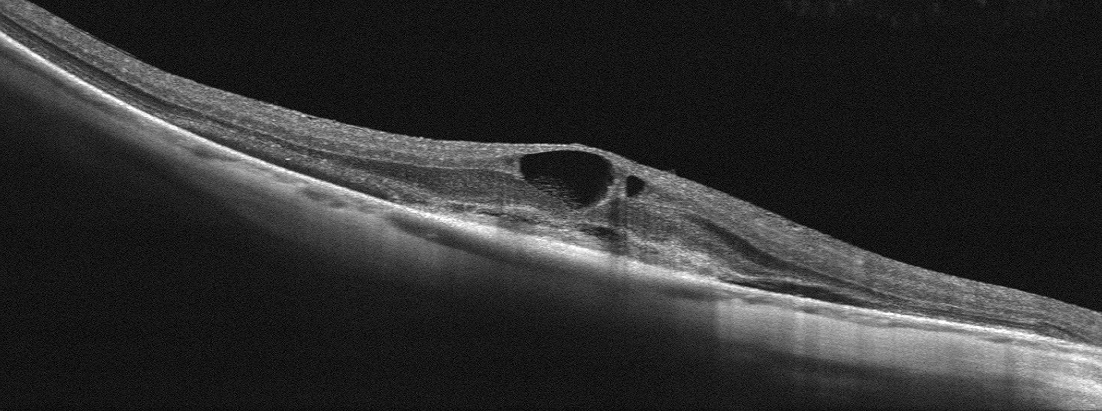

Retinal OCT B-scan; acquired on an Optovue Avanti RTVue XR — Macular OCT: age-related macular degeneration (AMD).